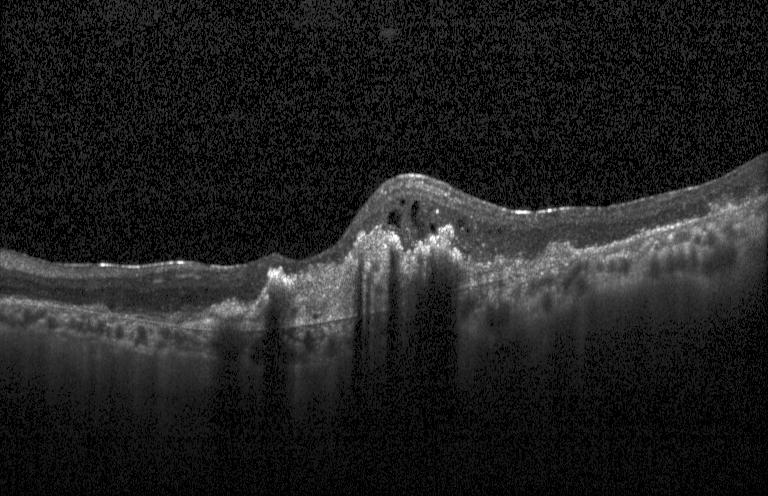

OCT line scan, horizontal scan through the fovea, spectral-domain optical coherence tomography, Heidelberg Spectralis OCT system.
The scan shows CNV.